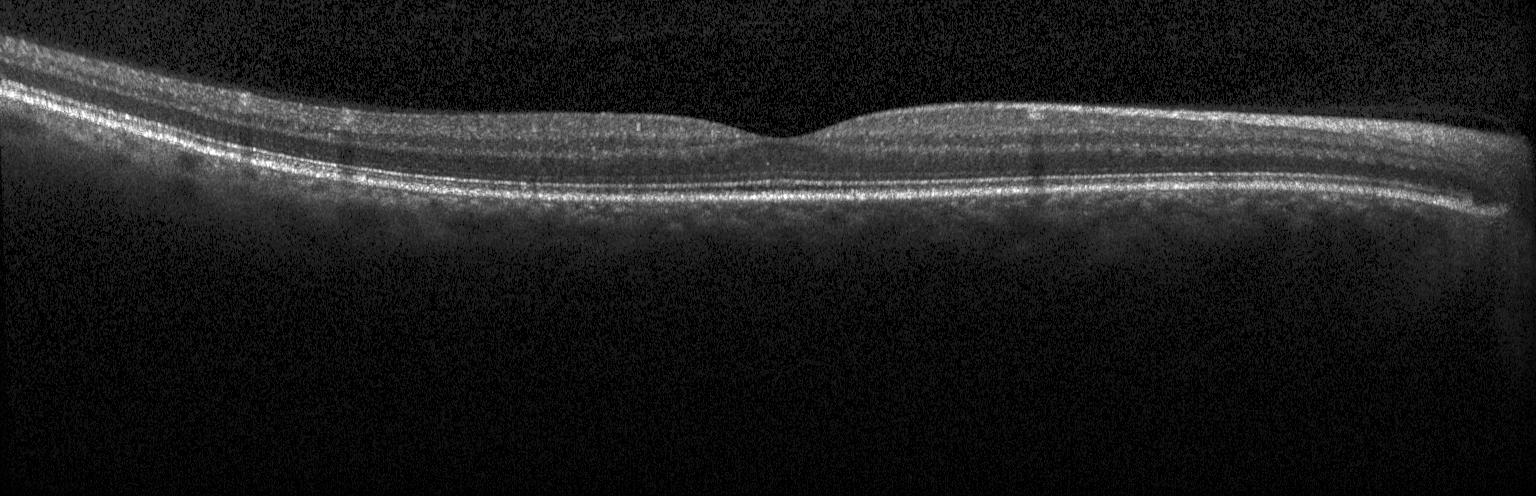 Retinal OCT B-scan, spectral-domain optical coherence tomography, through the macula, Heidelberg Spectralis — Finding: neither choroidal neovascularization, diabetic macular edema, nor drusen.